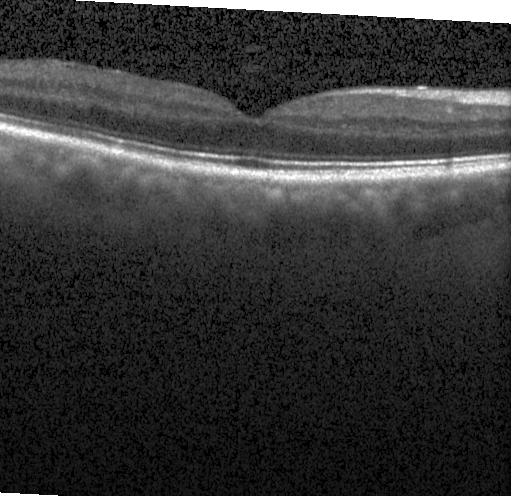 OCT B-scan; instrument: Heidelberg Spectralis; spectral-domain OCT; fovea-centered. Impression: no CNV, DME, or drusen.